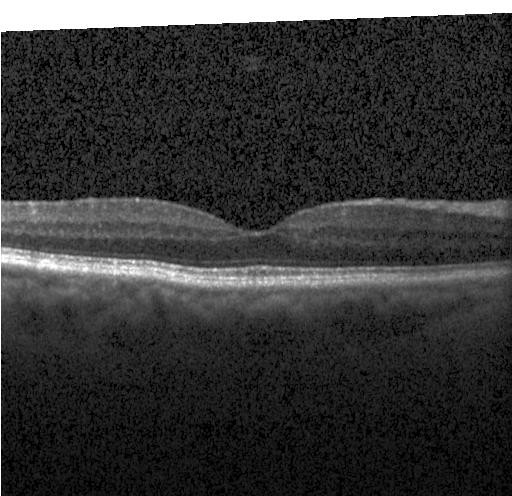

Diagnosis: no choroidal neovascularization, diabetic macular edema, or drusen.